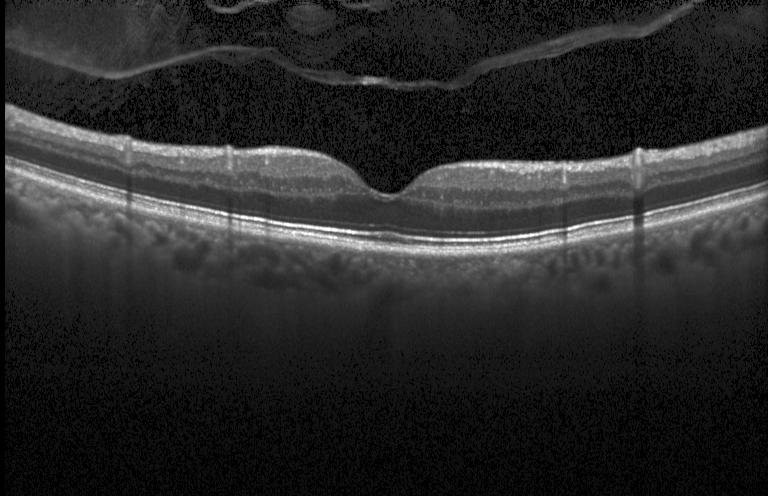

Neither choroidal neovascularization, diabetic macular edema, nor drusen.